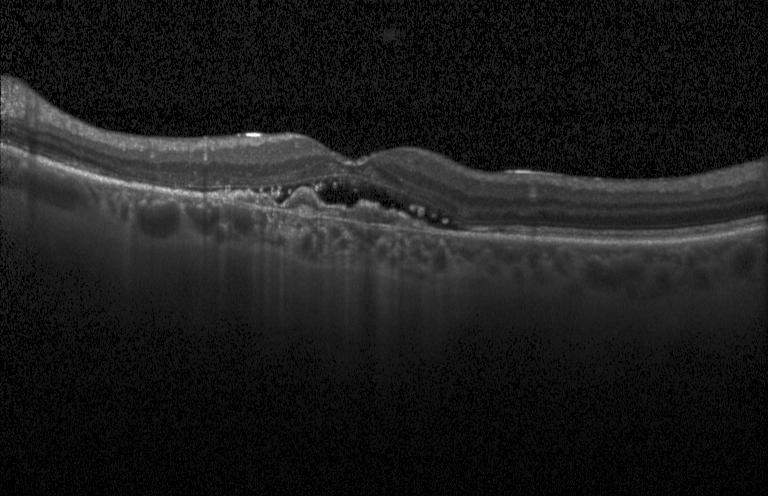 Macular OCT: a choroidal neovascular membrane.